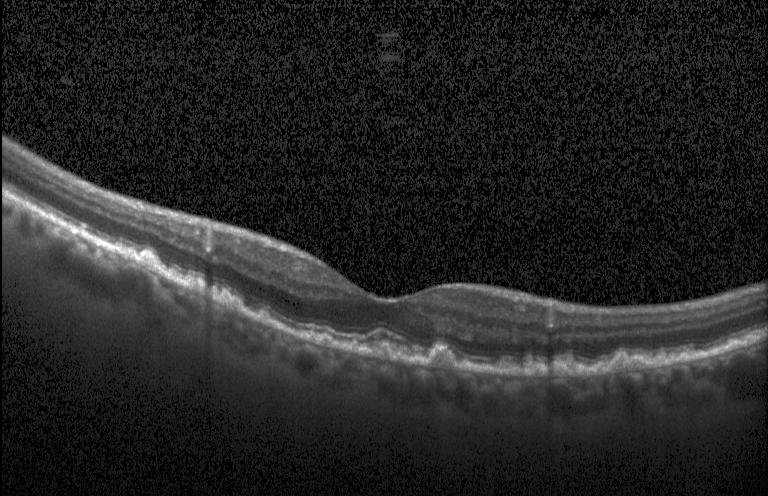

OCT finding: sub-RPE drusenoid deposits.